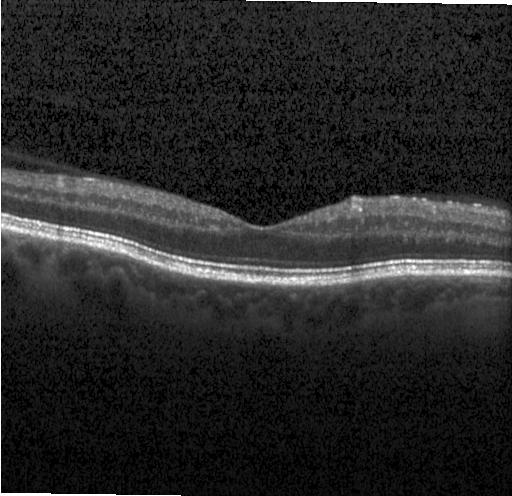

Impression: no choroidal neovascularization, diabetic macular edema, or drusen.